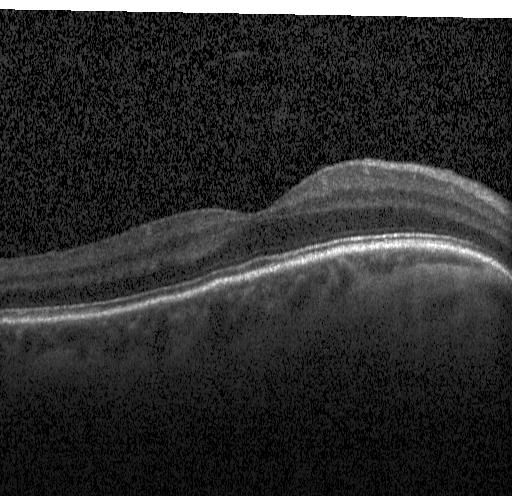
No choroidal neovascularization, diabetic macular edema, or drusen.